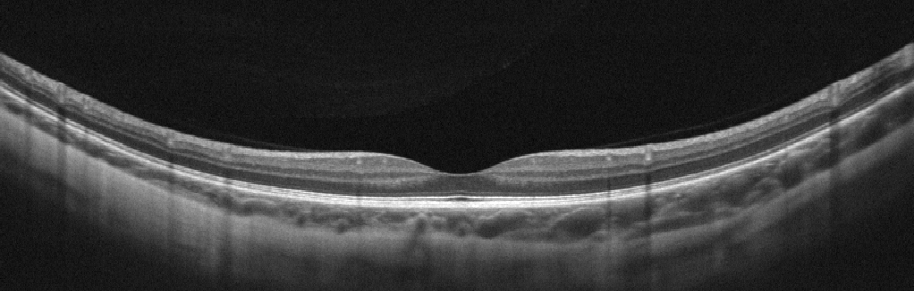

OCT line scan — Diagnosis: no evidence of AMD, DME, ERM, RAO, RVO, or VID.